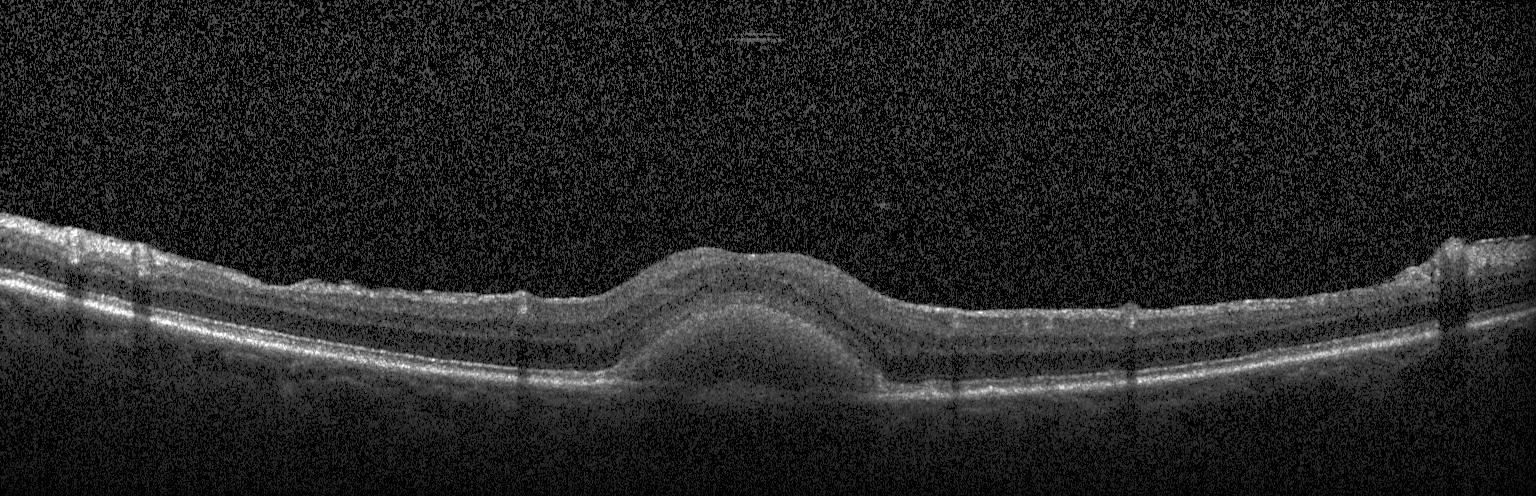

Centered on the fovea, SD-OCT, Heidelberg Spectralis, optical coherence tomography B-scan.
This B-scan demonstrates a choroidal neovascular membrane.